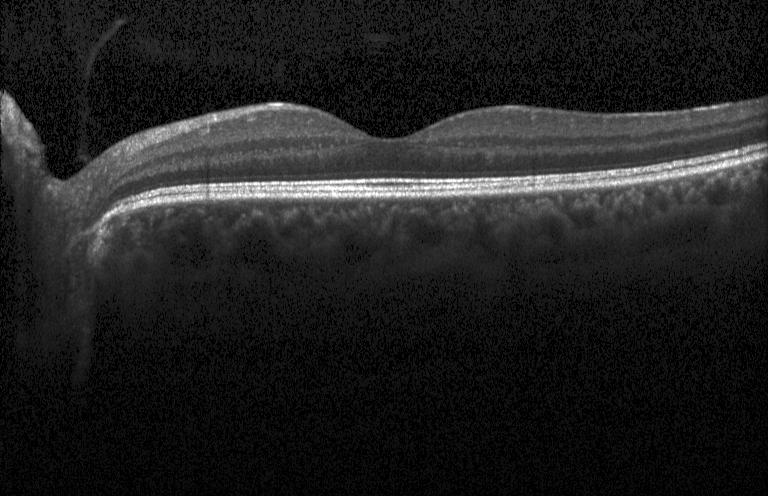
Macular OCT: no evidence of choroidal neovascularization, diabetic macular edema, or drusen.